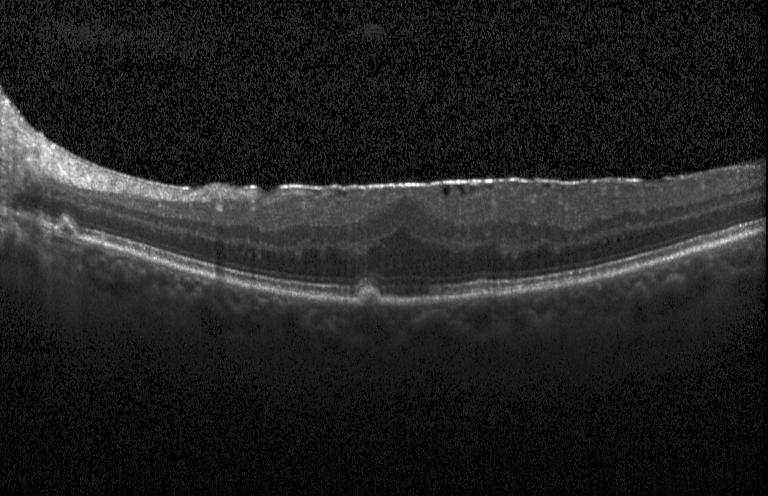

Finding: drusen.